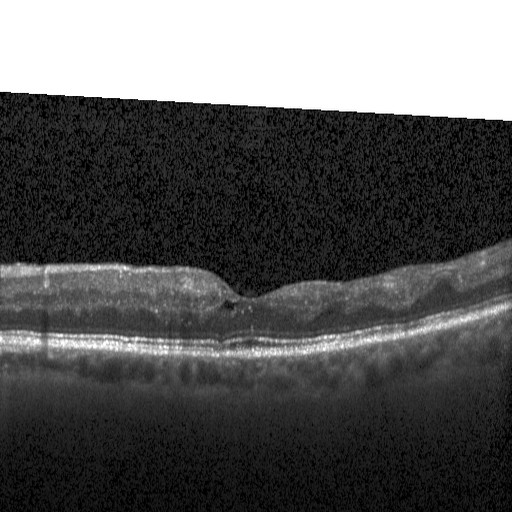

Heidelberg Spectralis OCT system, SD-OCT, horizontal scan through the fovea, optical coherence tomography scan — Finding: diabetic macular edema (DME).